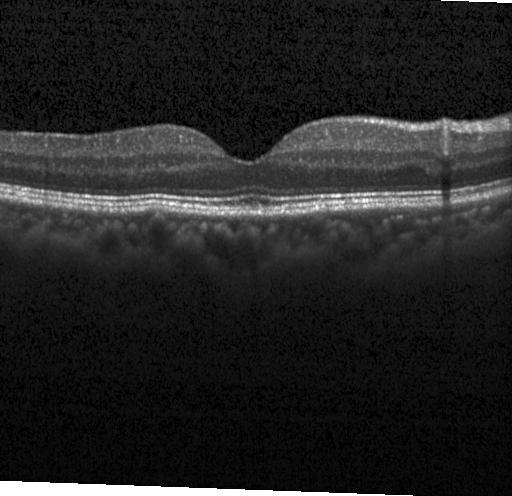 OCT B-scan. OCT finding: no CNV, no DME, and no drusen.